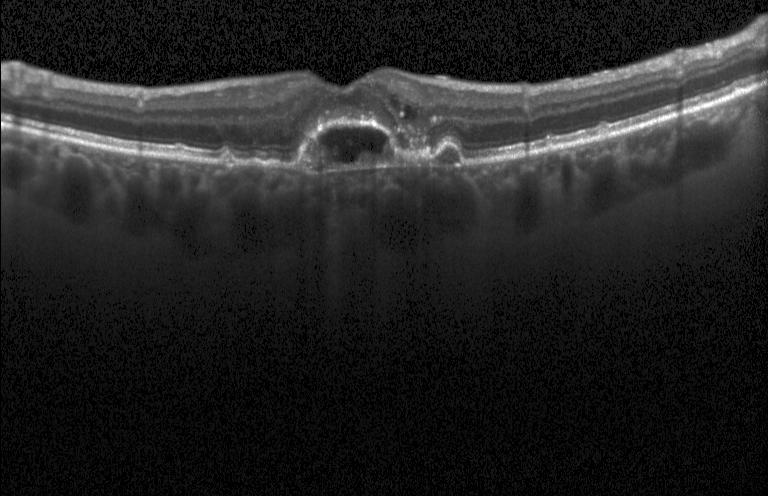

Retinal OCT B-scan. Macular scan.
Impression: a choroidal neovascular membrane.